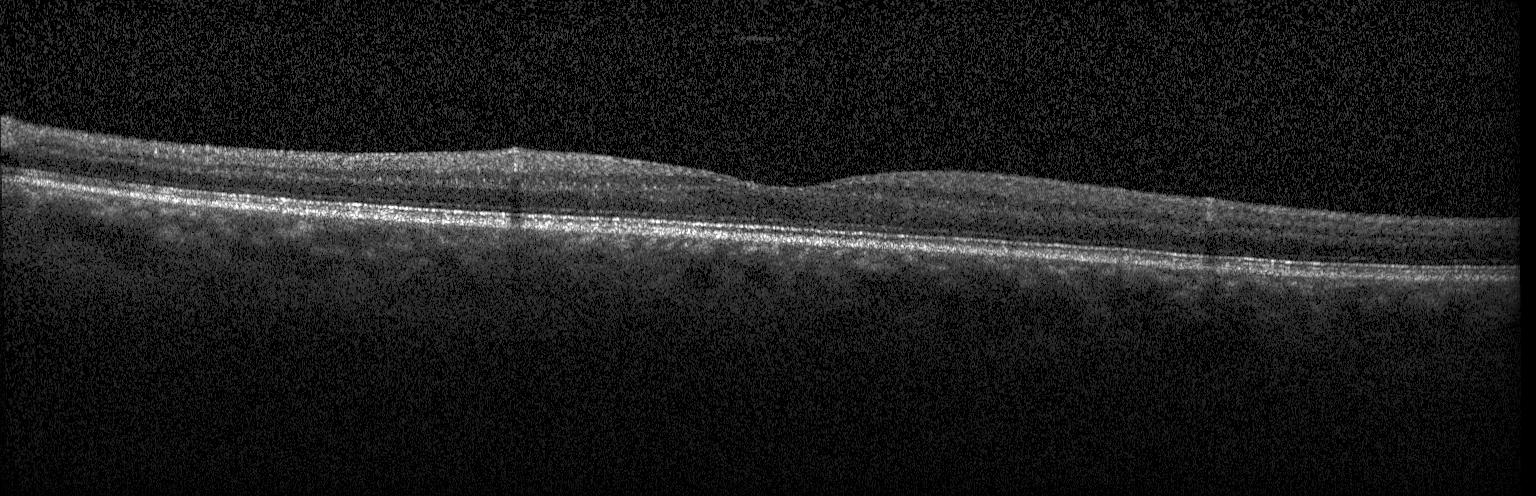 Retinal OCT cross-section. Spectral-domain OCT. Heidelberg Spectralis OCT system. Through the macula — Finding: no evidence of CNV, DME, or drusen.